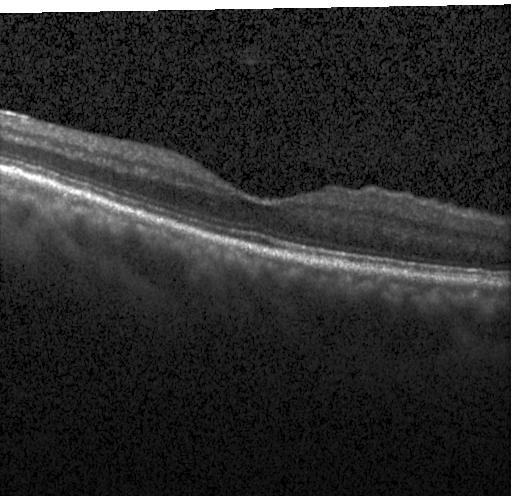 Spectral-domain optical coherence tomography, OCT B-scan — Diagnosis: no choroidal neovascularization, no diabetic macular edema, and no drusen.